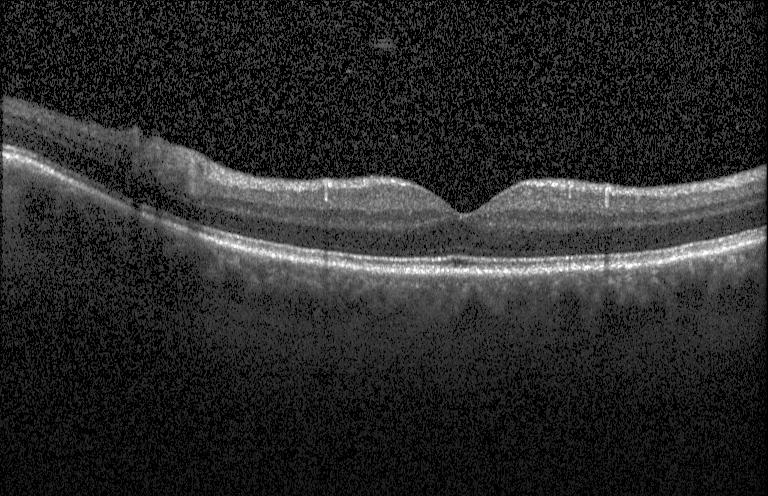
OCT finding: no CNV, DME, or drusen.